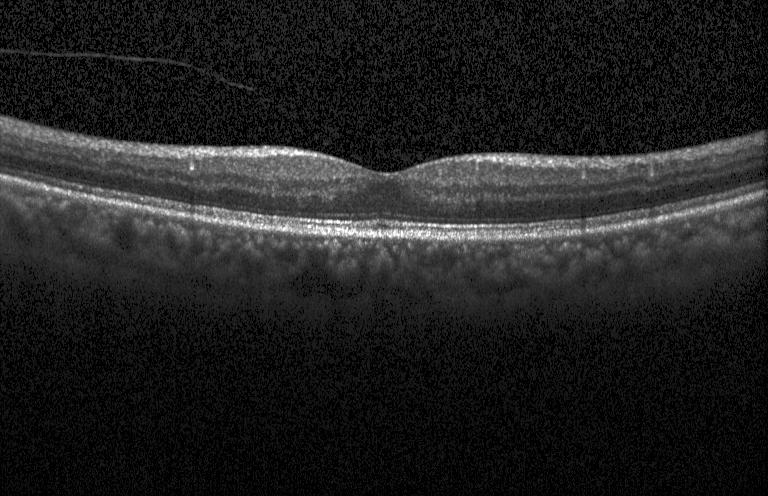 Centered on the fovea · spectral-domain OCT · optical coherence tomography scan · Heidelberg Spectralis OCT system. This B-scan demonstrates no evidence of CNV, DME, or drusen.